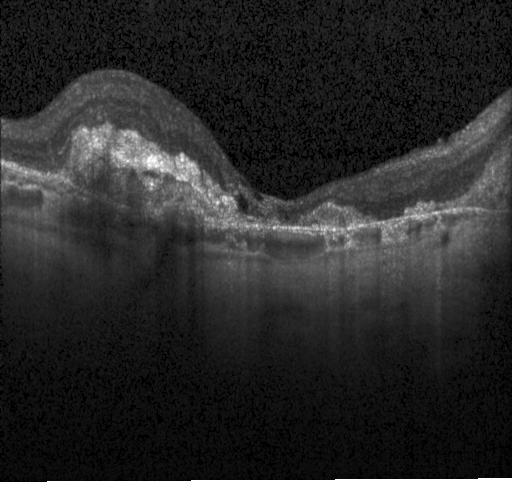

Diagnosis: choroidal neovascularization (CNV).